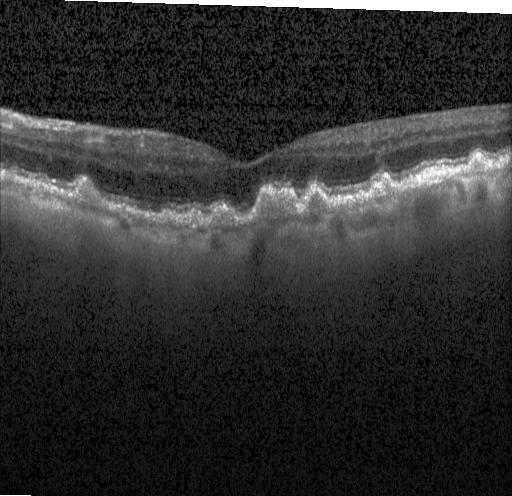
Optical coherence tomography B-scan.
Finding: sub-RPE drusenoid deposits.